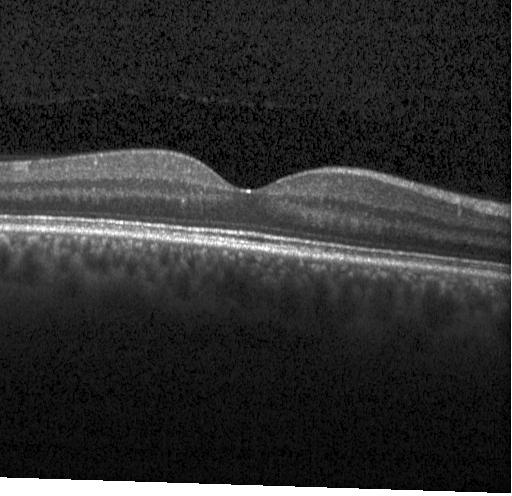
Optical coherence tomography scan — Assessment: no evidence of CNV, DME, or drusen.